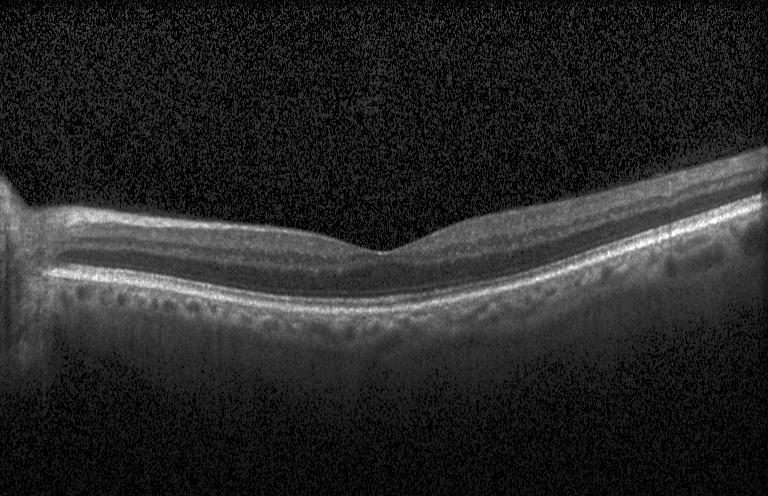
Optical coherence tomography B-scan. Heidelberg Spectralis. Diagnosis: neither CNV, DME, nor drusen.